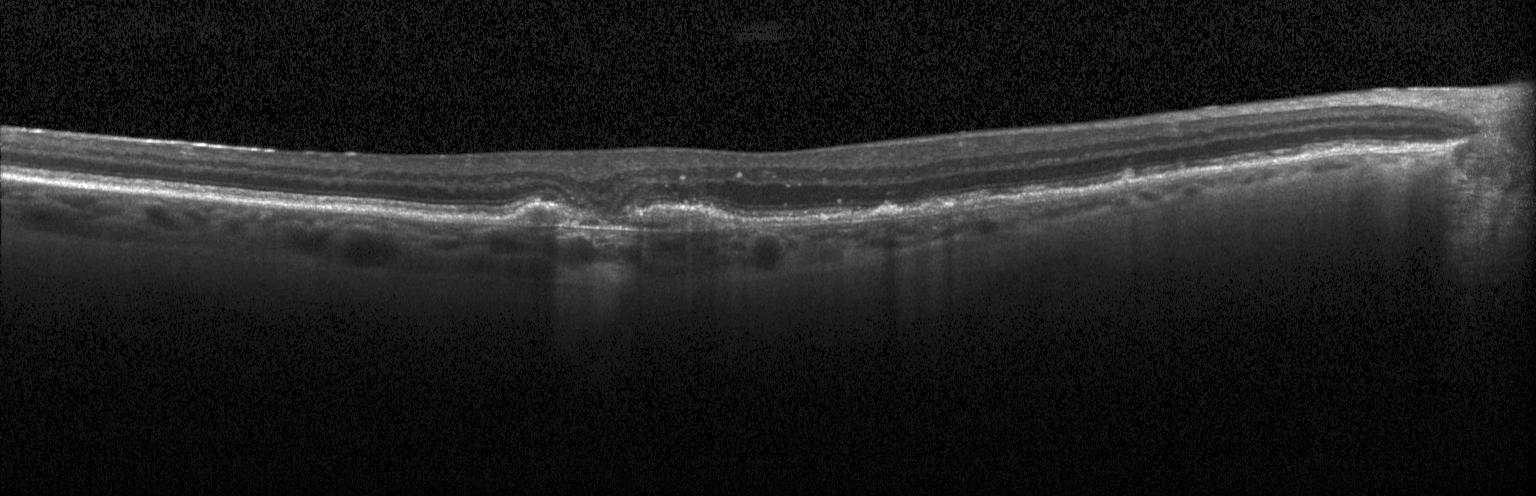

Fovea-centered; spectral-domain OCT; optical coherence tomography scan; acquired on a Heidelberg Spectralis
Diagnosis: CNV.